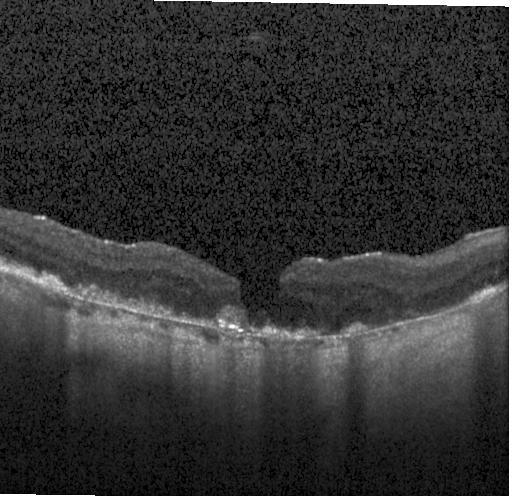

Spectral-domain OCT. Optical coherence tomography scan. Impression: CNV.